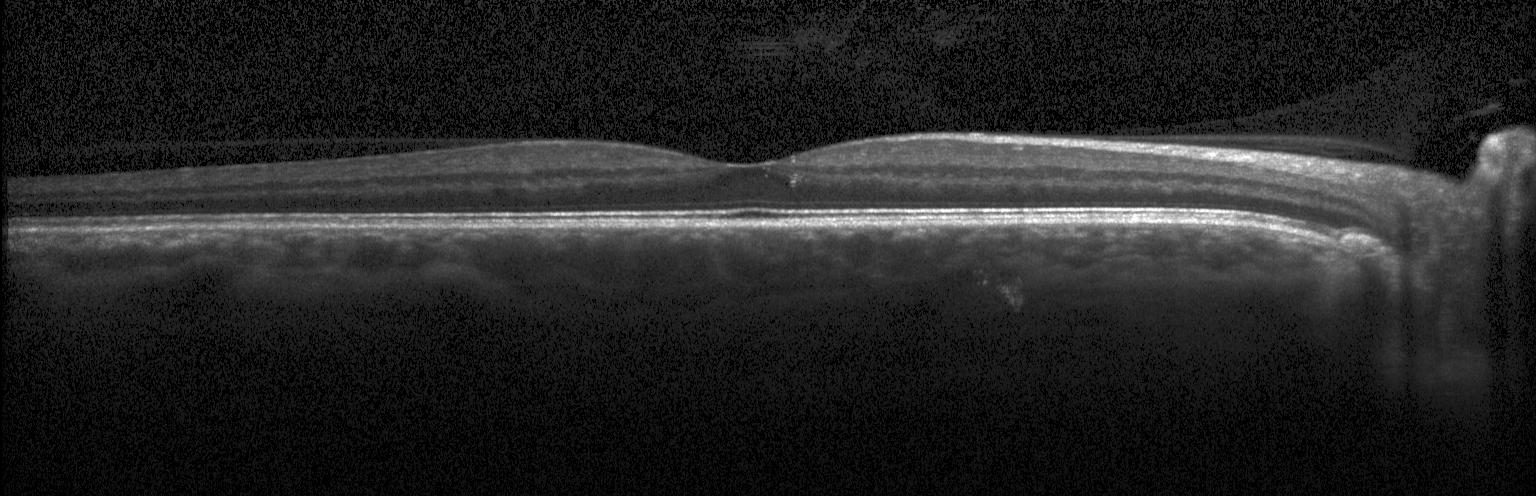

Instrument: Heidelberg Spectralis. Retinal OCT cross-section
Dx: neither choroidal neovascularization, diabetic macular edema, nor drusen.